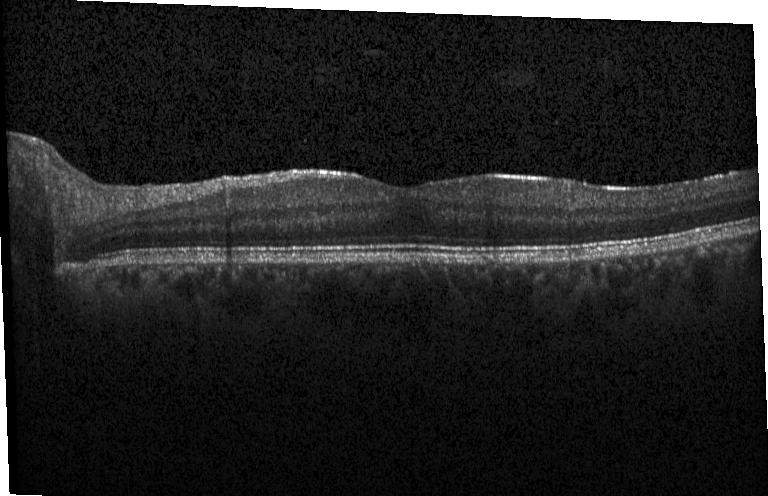

Spectral-domain OCT B-scan: no CNV, DME, or drusen.